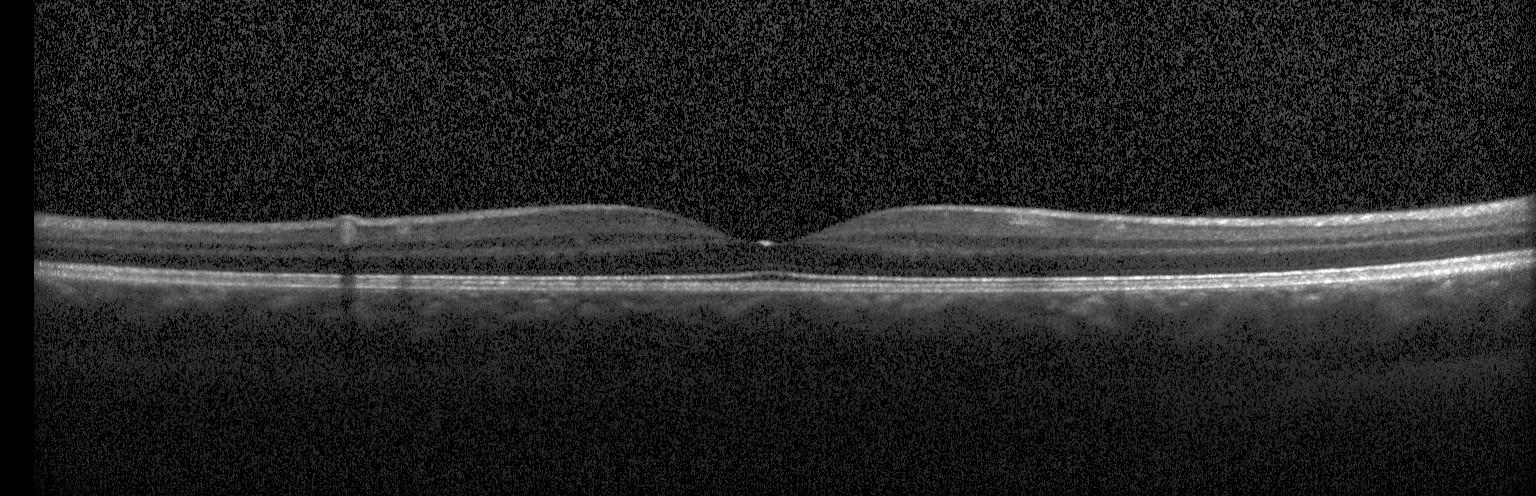

Horizontal scan through the fovea · OCT B-scan · Heidelberg Spectralis OCT system · spectral-domain optical coherence tomography
Finding: neither choroidal neovascularization, diabetic macular edema, nor drusen.